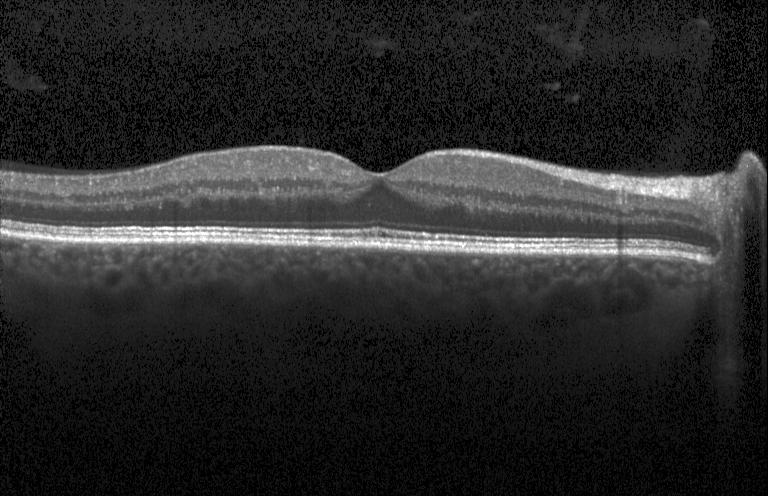

Diagnosis: no choroidal neovascularization, no diabetic macular edema, and no drusen.